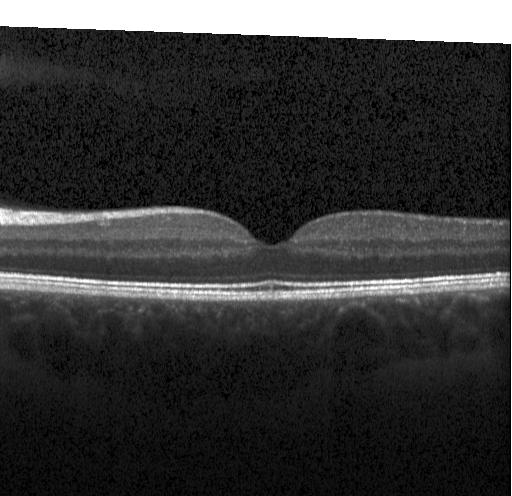 Fovea-centered; retinal OCT cross-section; spectral-domain OCT
Finding: no choroidal neovascularization, diabetic macular edema, or drusen.